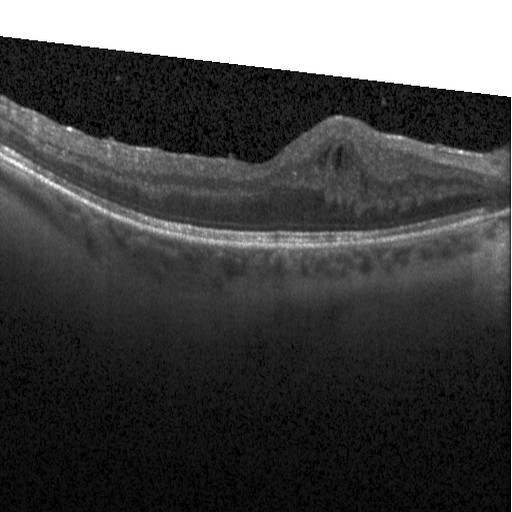

OCT scan showing diabetic macular edema (DME).